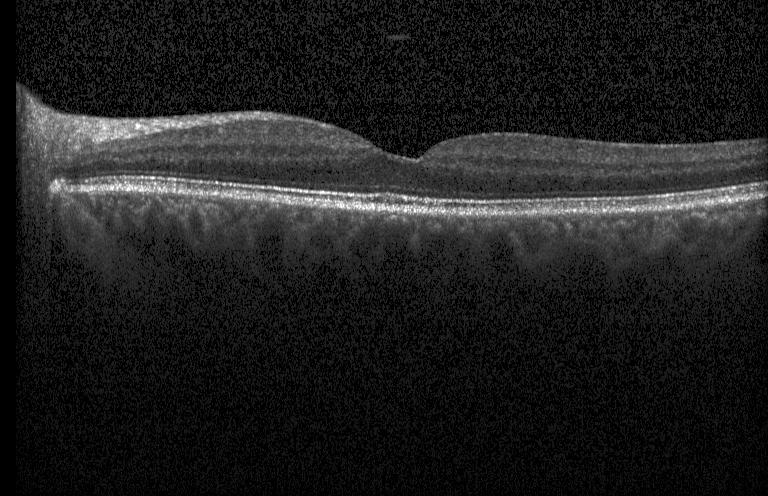 This B-scan demonstrates no choroidal neovascularization, no diabetic macular edema, and no drusen.